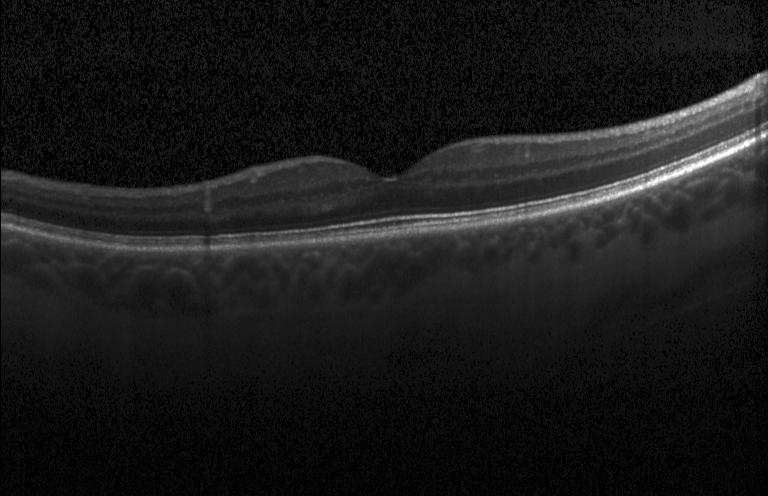

Finding: no choroidal neovascularization, diabetic macular edema, or drusen.